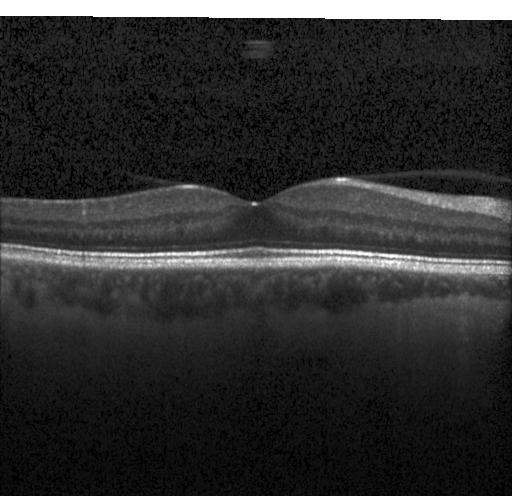

OCT B-scan. Finding: neither choroidal neovascularization, diabetic macular edema, nor drusen.